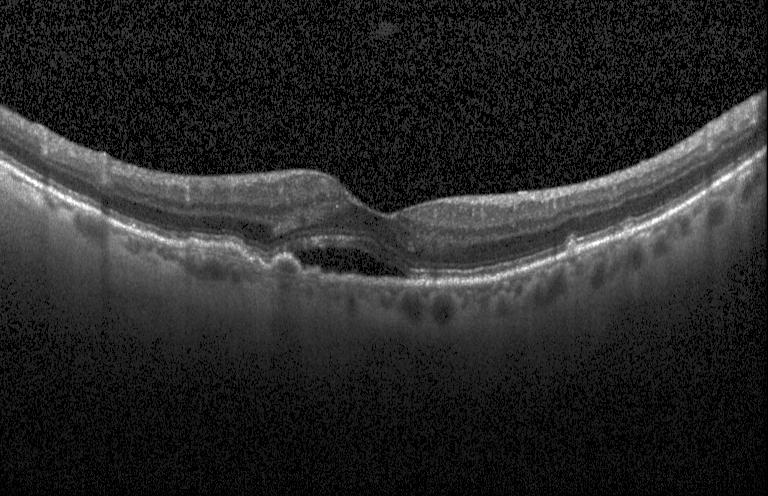
OCT line scan — Dx: CNV.